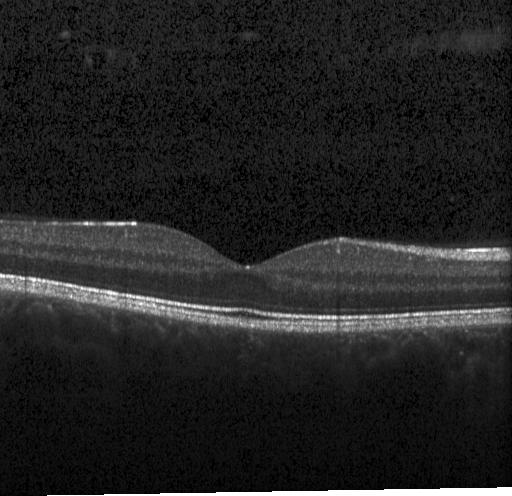

Horizontal scan through the fovea, SD-OCT, retinal OCT B-scan. Finding: no choroidal neovascularization, diabetic macular edema, or drusen.